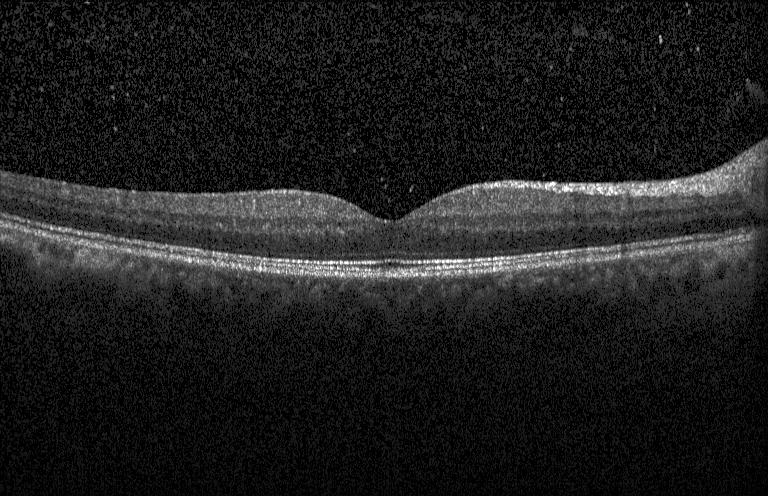 Optical coherence tomography scan. Assessment: no choroidal neovascularization, diabetic macular edema, or drusen.